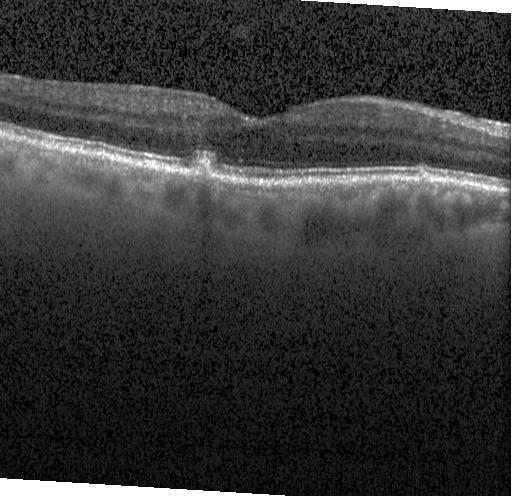

Impression: sub-RPE drusenoid deposits.